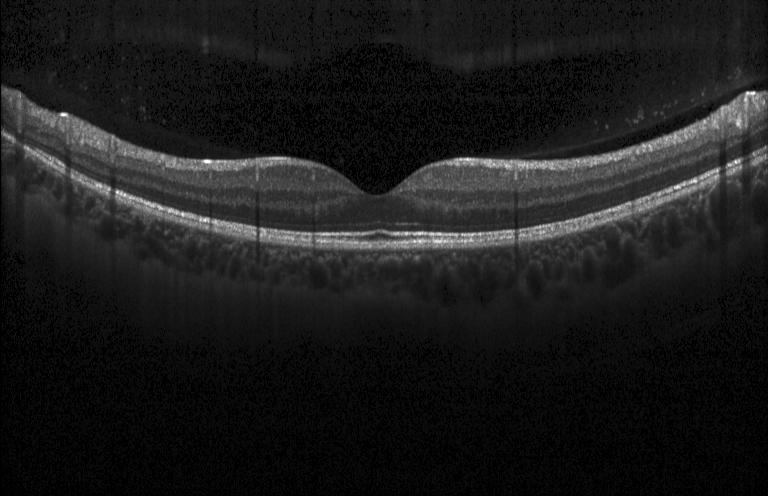 Heidelberg Spectralis OCT system; OCT line scan; macular scan.
This B-scan demonstrates no choroidal neovascularization, diabetic macular edema, or drusen.